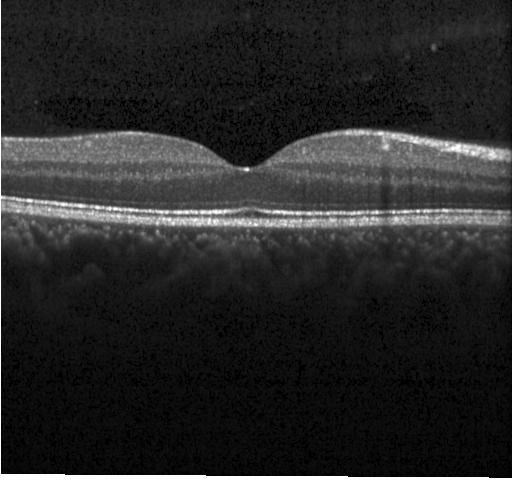

No choroidal neovascularization, no diabetic macular edema, and no drusen.